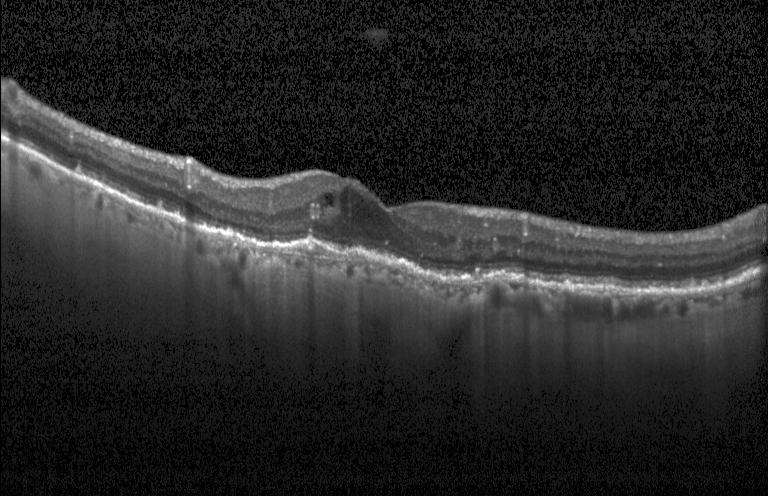 Impression: CNV.